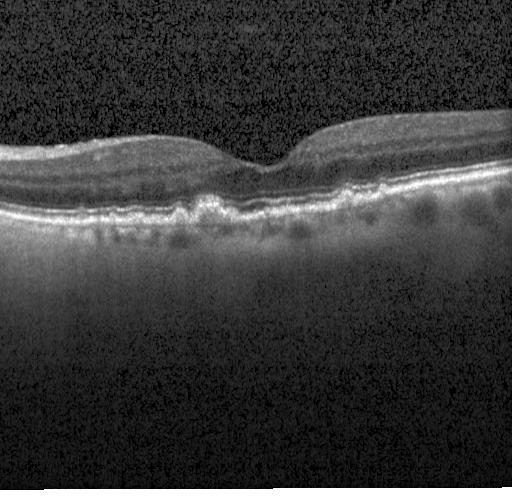

Fovea-centered; retinal OCT cross-section; spectral-domain OCT; instrument: Heidelberg Spectralis — Impression: drusen.